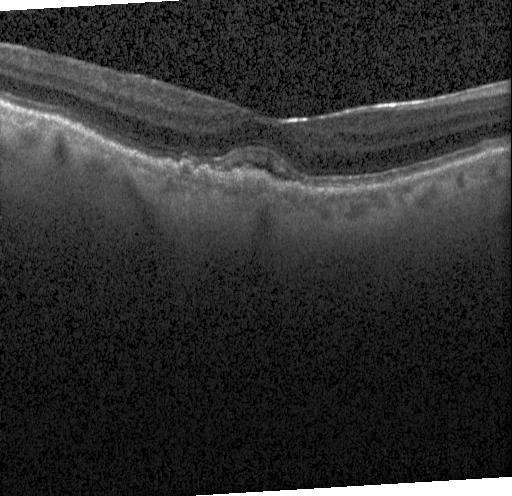 Assessment: a choroidal neovascular membrane.